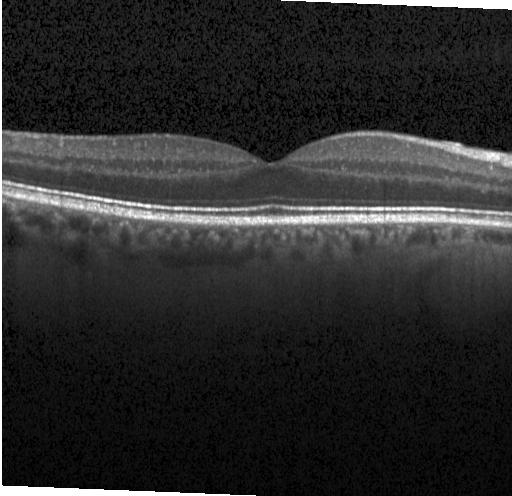

OCT line scan. Horizontal scan through the fovea. SD-OCT
Impression: no choroidal neovascularization, no diabetic macular edema, and no drusen.